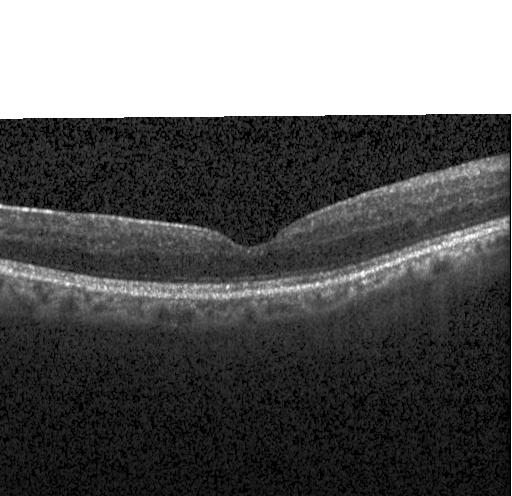
Retinal OCT cross-section showing no choroidal neovascularization, no diabetic macular edema, and no drusen.